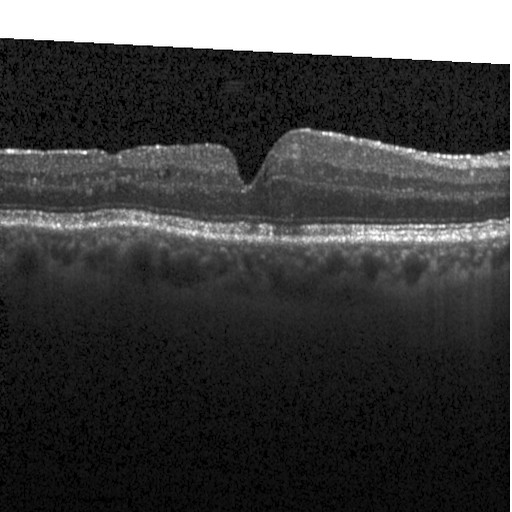 Acquired on a Heidelberg Spectralis; centered on the fovea; retinal OCT cross-section; spectral-domain OCT — Diagnosis: diabetic macular edema (DME).